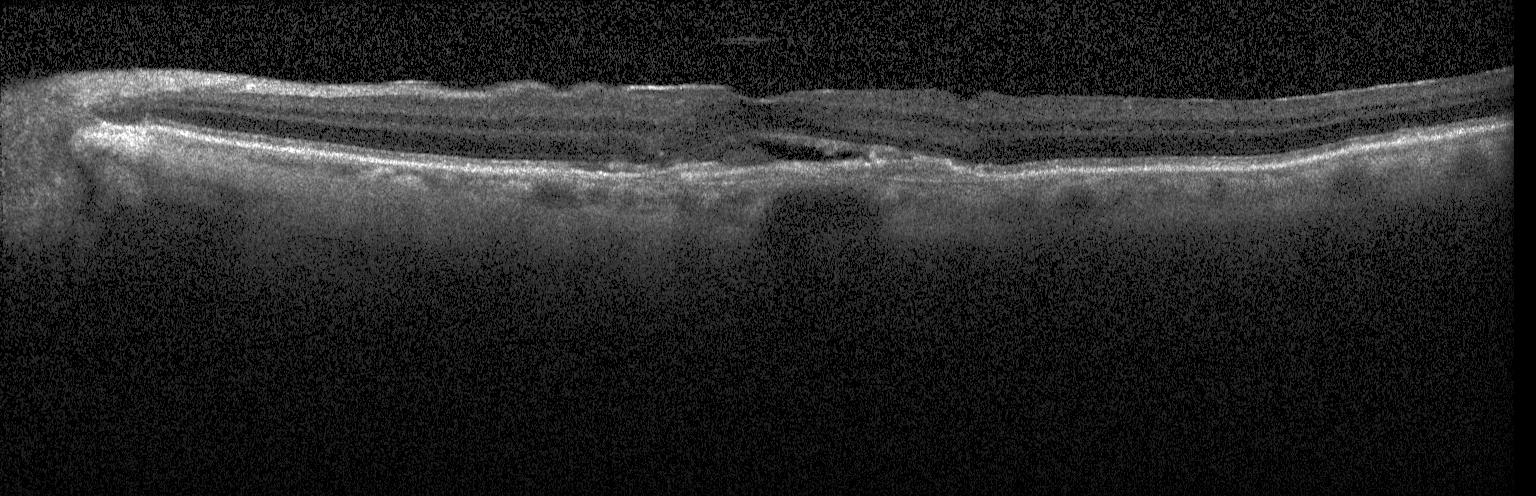 This B-scan demonstrates choroidal neovascularization.